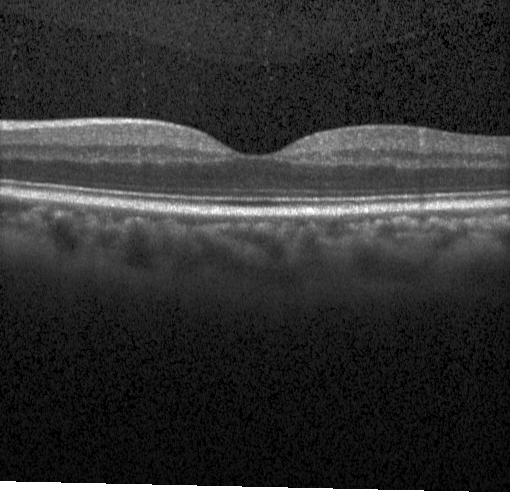 Through the macula, OCT B-scan, spectral-domain optical coherence tomography. Diagnosis: no choroidal neovascularization, no diabetic macular edema, and no drusen.